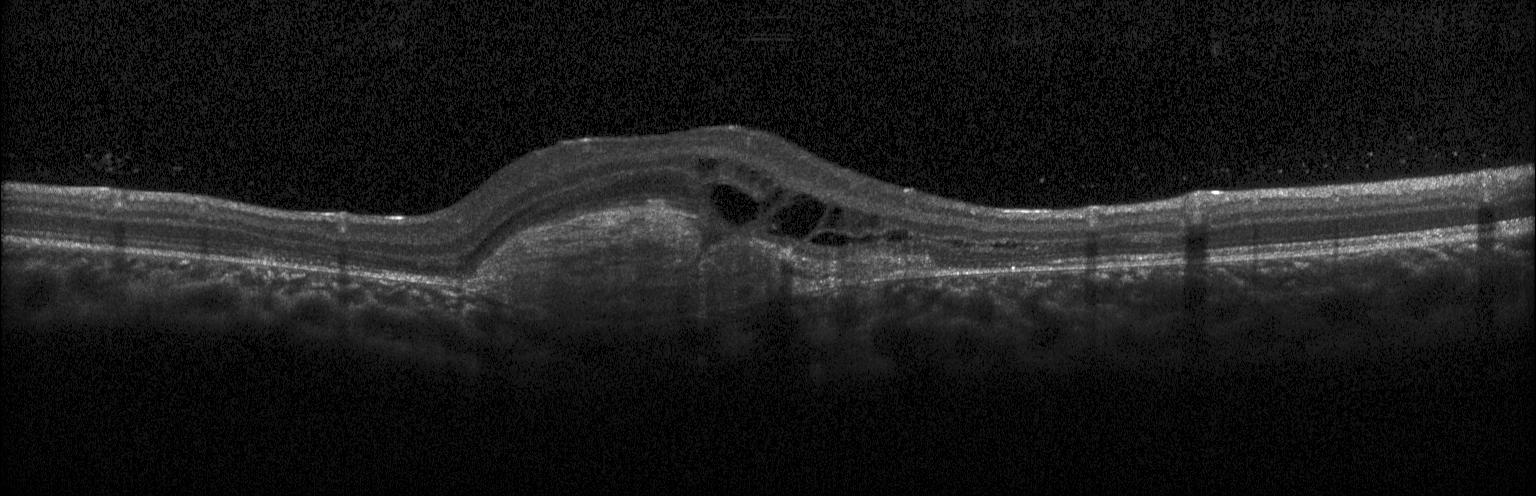 OCT B-scan showing a choroidal neovascular membrane.